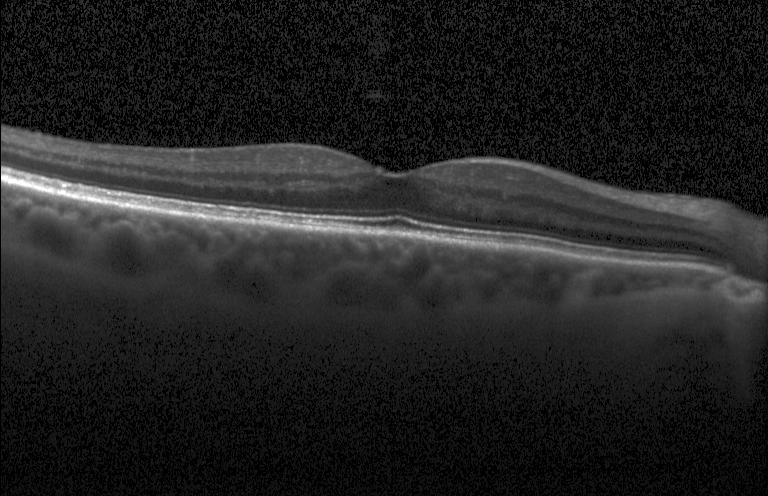
Macular OCT: no choroidal neovascularization, diabetic macular edema, or drusen.